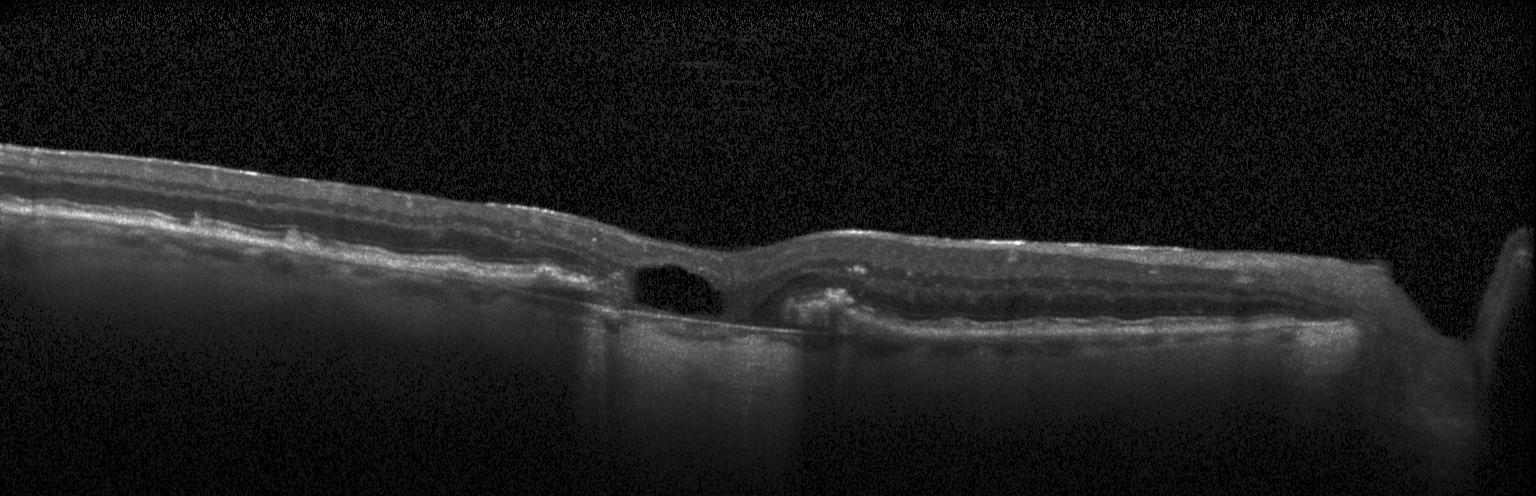 Assessment: a choroidal neovascular membrane.